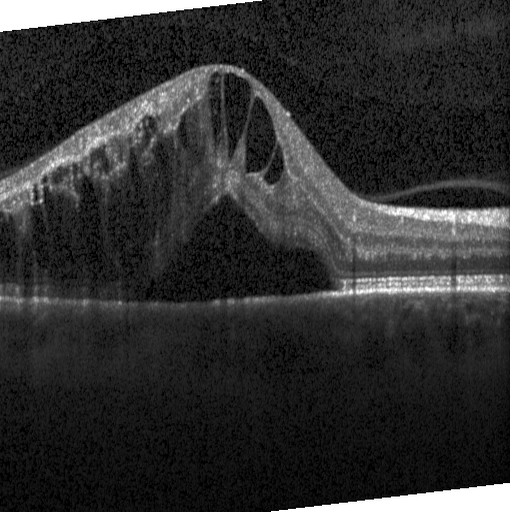

Macular scan, Heidelberg Spectralis OCT system, retinal OCT B-scan, spectral-domain OCT
Dx: DME.